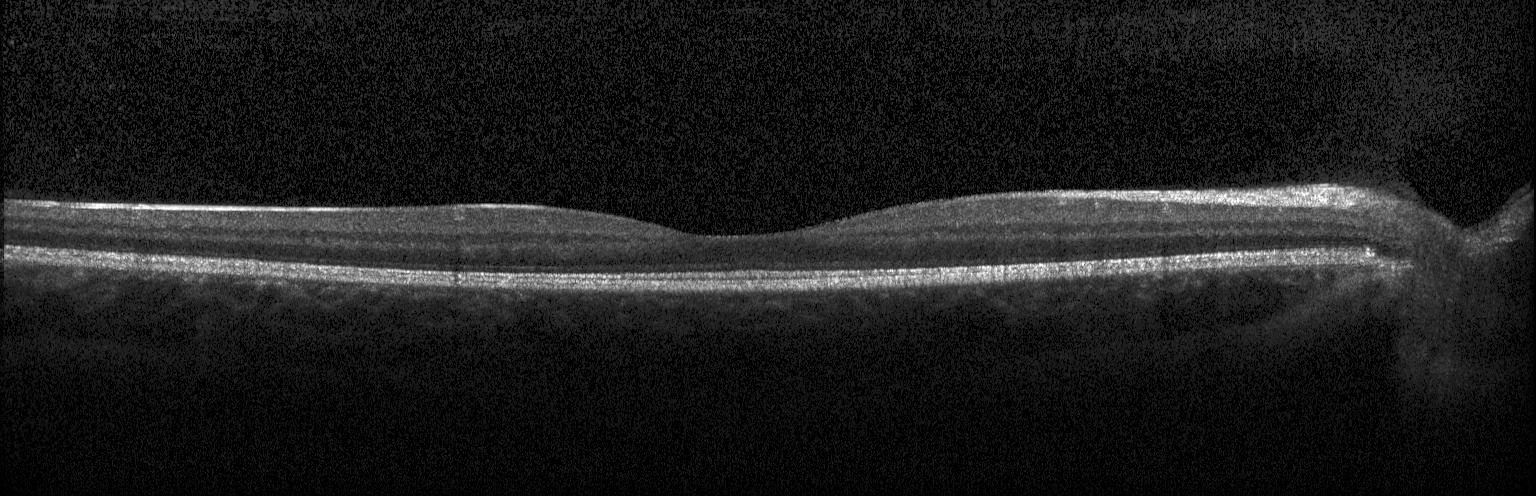
Assessment: no choroidal neovascularization, diabetic macular edema, or drusen.